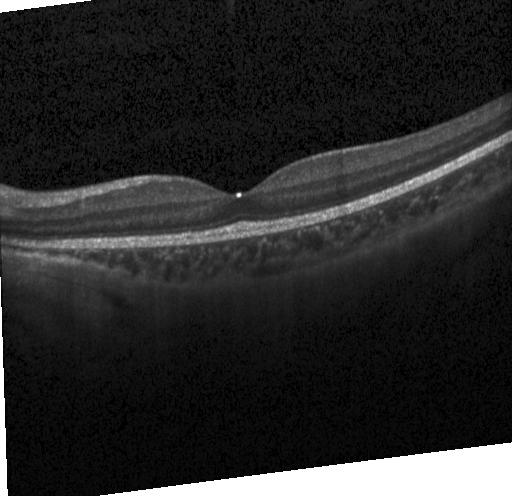 Assessment: neither choroidal neovascularization, diabetic macular edema, nor drusen.